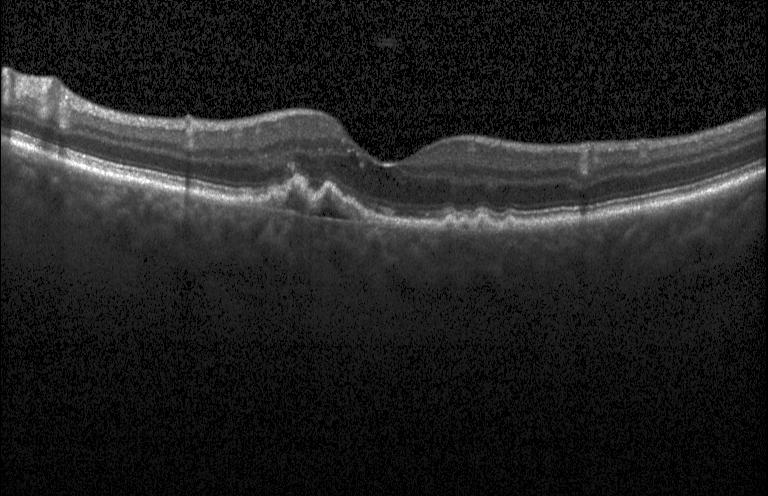
Macular OCT demonstrating a choroidal neovascular membrane.